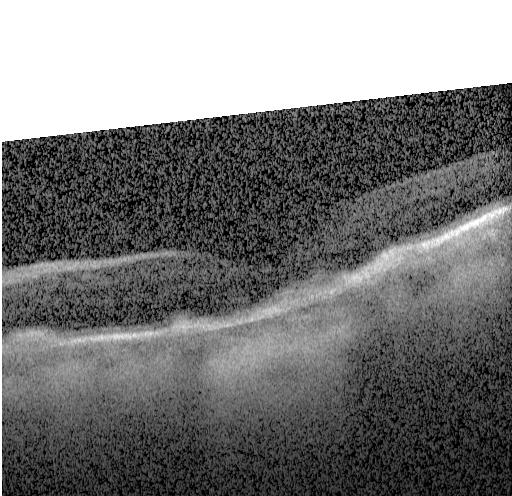 Spectral-domain OCT B-scan: a choroidal neovascular membrane.